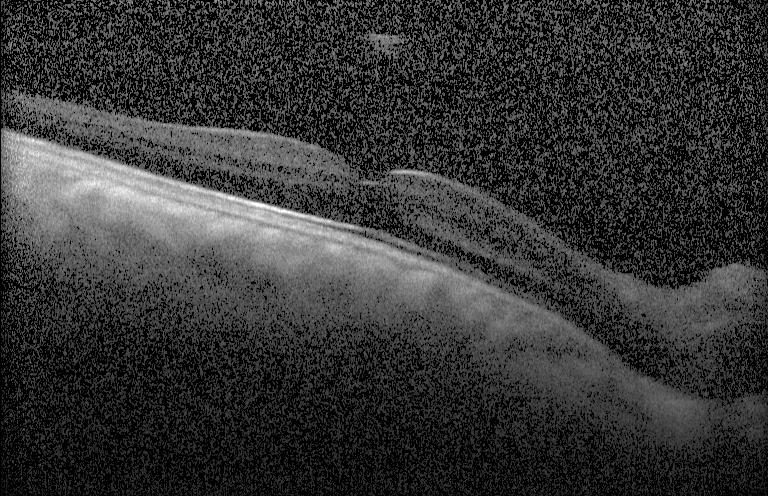
Optical coherence tomography scan
This B-scan demonstrates no choroidal neovascularization, no diabetic macular edema, and no drusen.